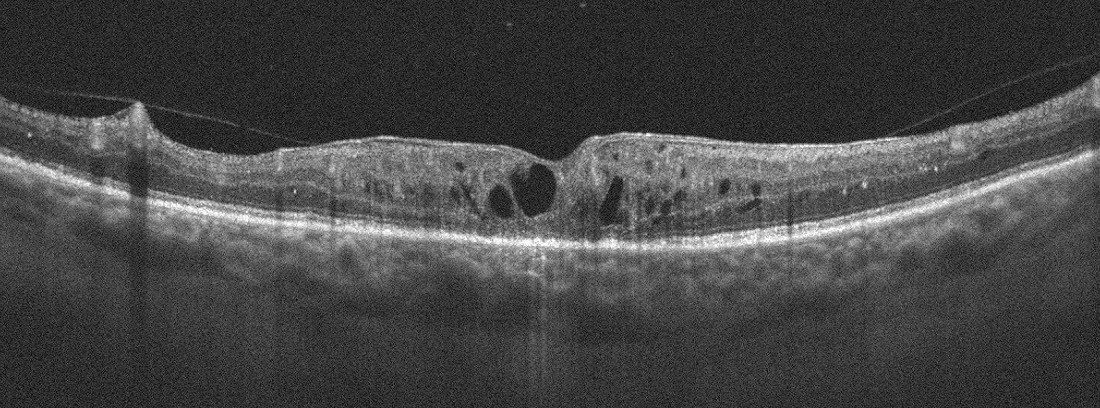

OCT B-scan; acquired on an Optovue Avanti RTVue XR — Diabetic macular edema (DME).